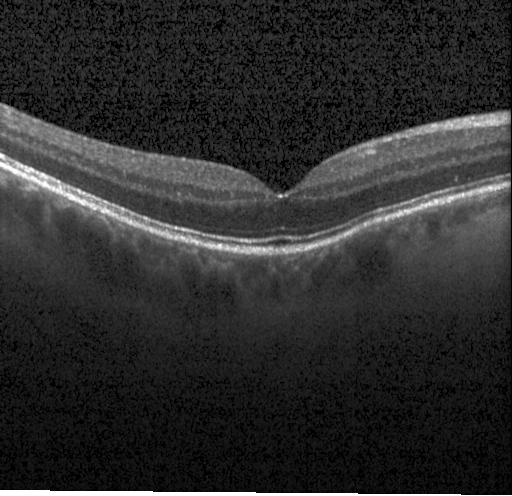
Optical coherence tomography B-scan.
Dx: no choroidal neovascularization, diabetic macular edema, or drusen.